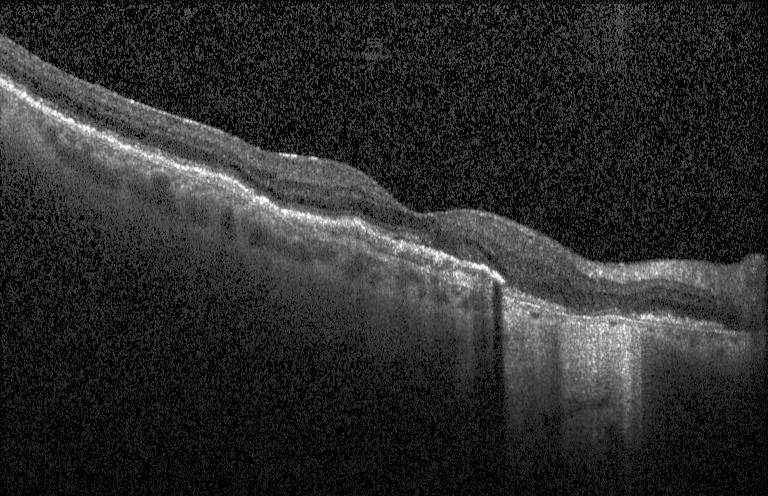
This B-scan demonstrates CNV.